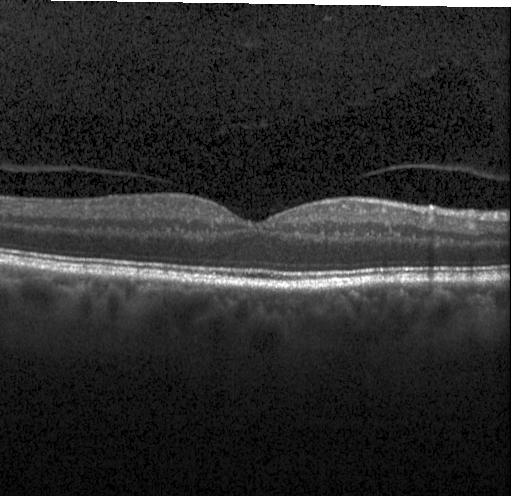 Retinal OCT B-scan. Through the macula. OCT finding: no CNV, no DME, and no drusen.